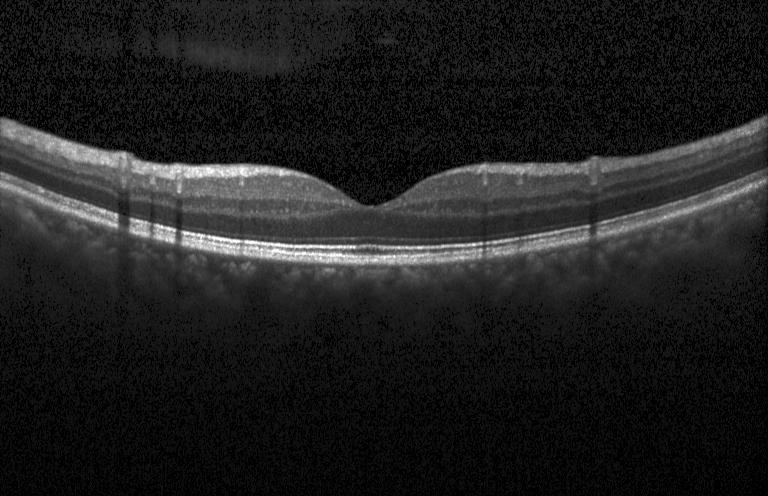
Through the macula; optical coherence tomography scan; SD-OCT
Impression: no CNV, DME, or drusen.